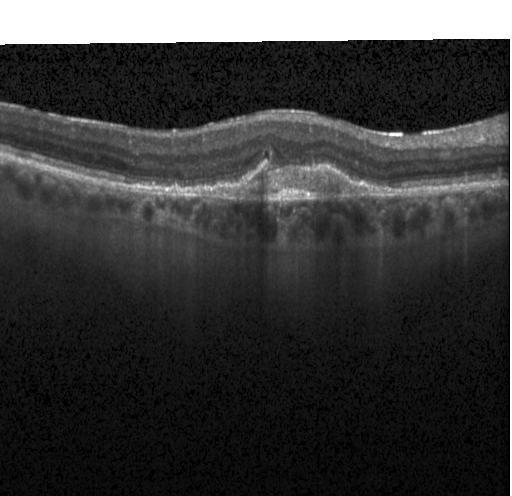

OCT B-scan.
Impression: a choroidal neovascular membrane.